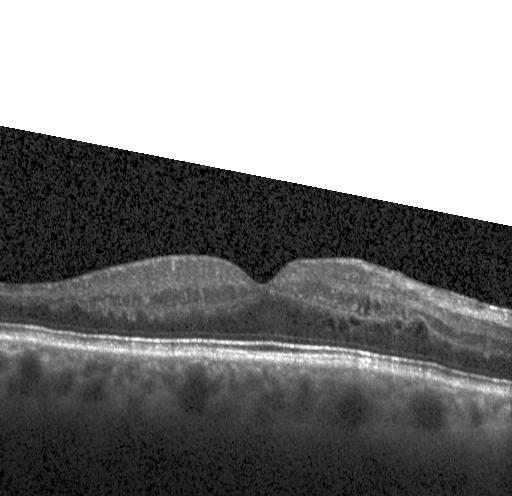 Optical coherence tomography scan.
This B-scan demonstrates diabetic macular edema (DME).